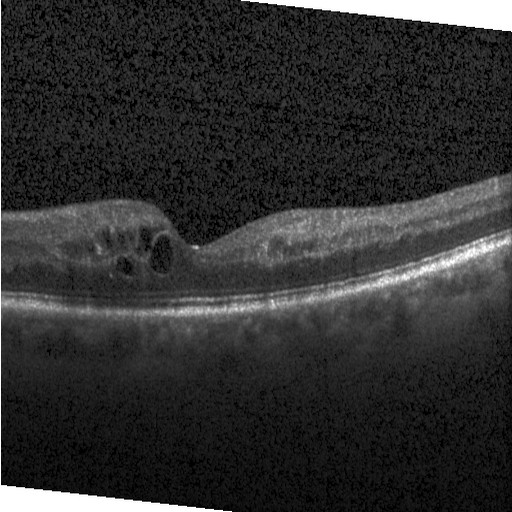

OCT finding: DME.